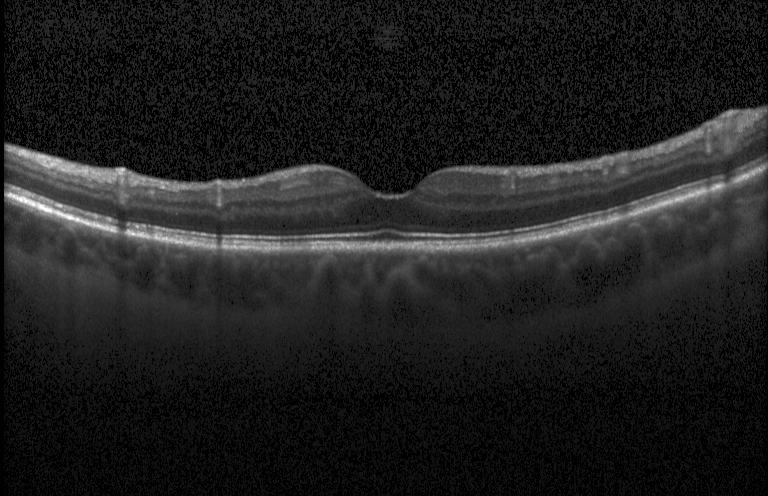 OCT B-scan, centered on the fovea.
Assessment: neither choroidal neovascularization, diabetic macular edema, nor drusen.